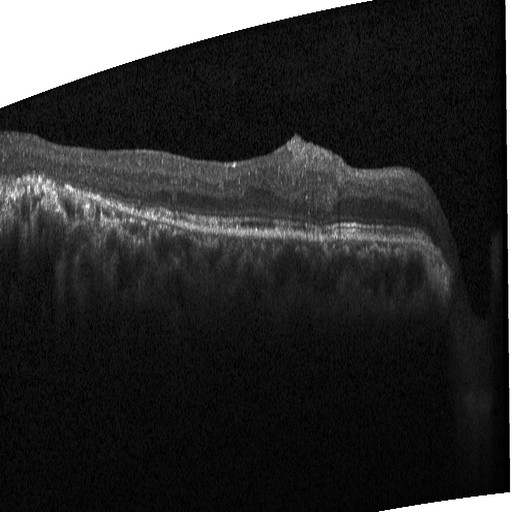 Macular scan · Heidelberg Spectralis · spectral-domain OCT · retinal OCT cross-section
Diagnosis: diabetic macular edema (DME).